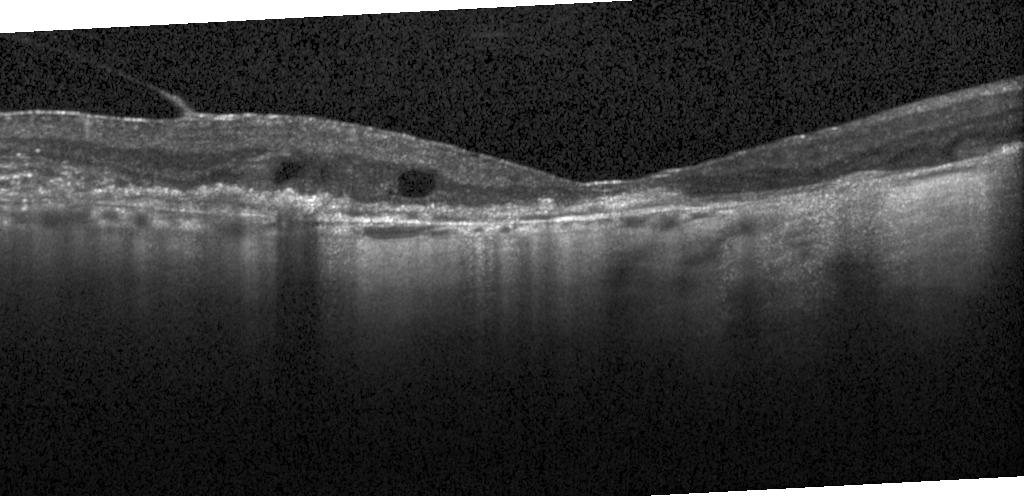 Retinal OCT B-scan. Impression: choroidal neovascularization.